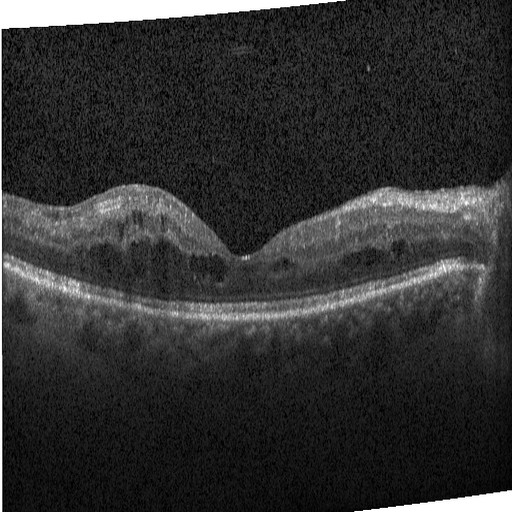
OCT B-scan. Diagnosis: diabetic macular edema.